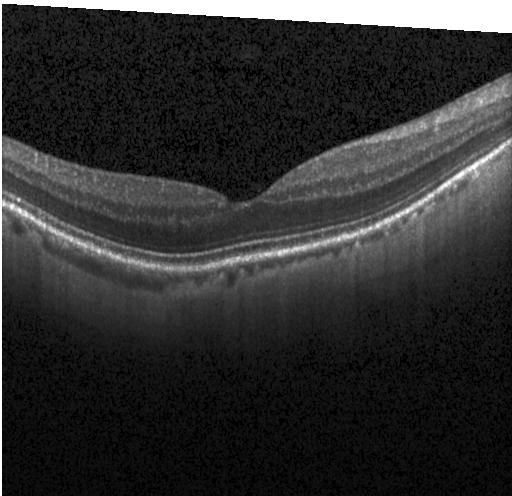 The scan shows no evidence of CNV, DME, or drusen.